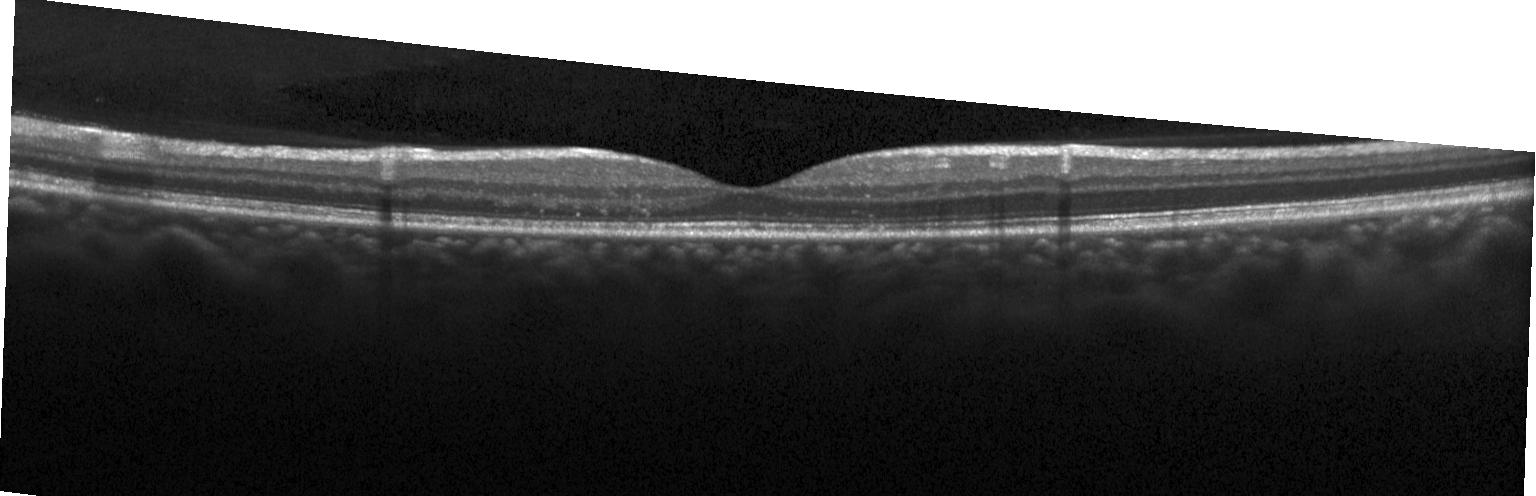

OCT B-scan. No CNV, no DME, and no drusen.